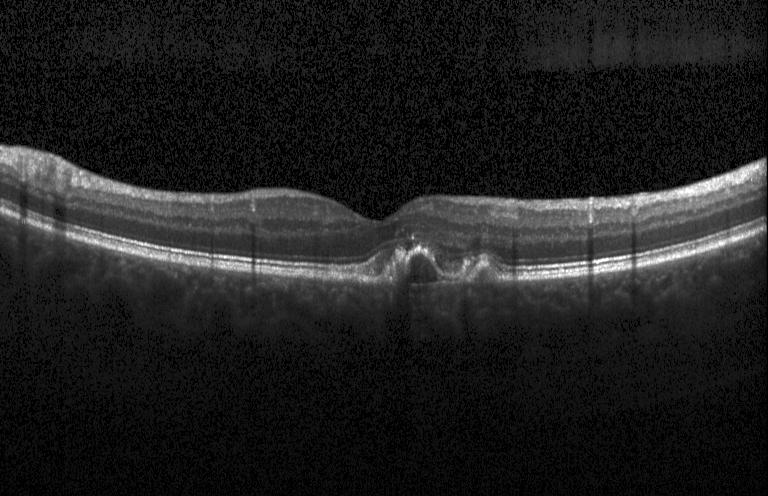
Assessment: choroidal neovascularization.